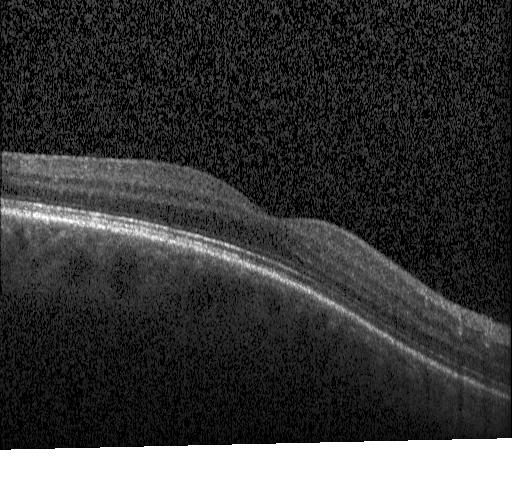 Retinal OCT B-scan. SD-OCT. Acquired on a Heidelberg Spectralis. No CNV, DME, or drusen.